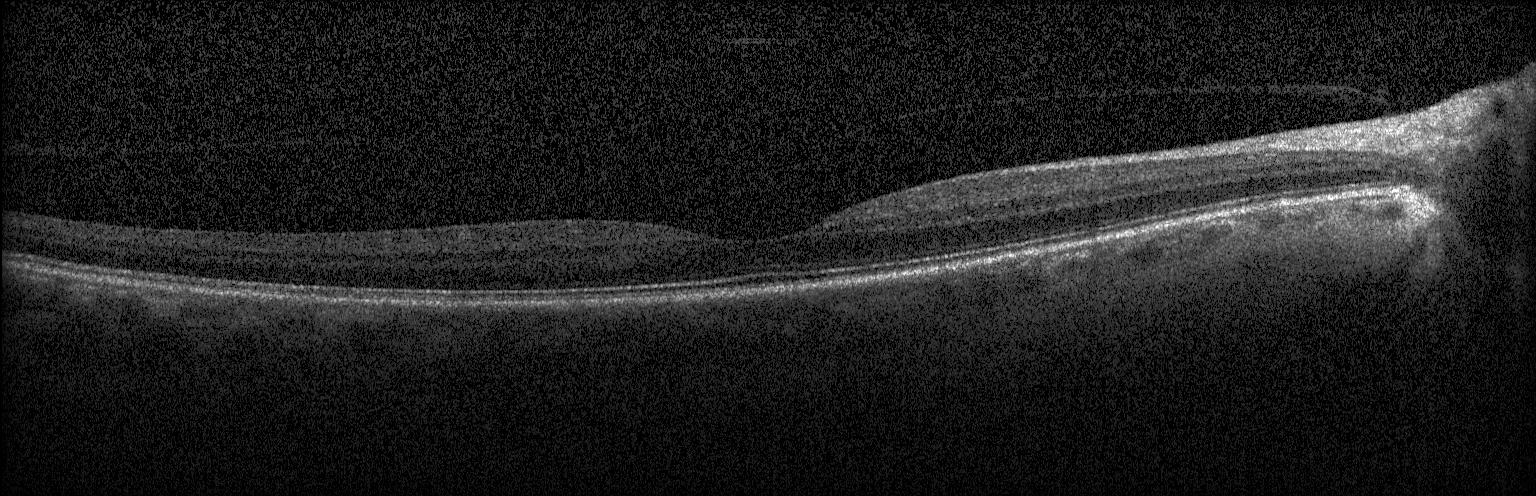

Macular OCT demonstrating no evidence of choroidal neovascularization, diabetic macular edema, or drusen.